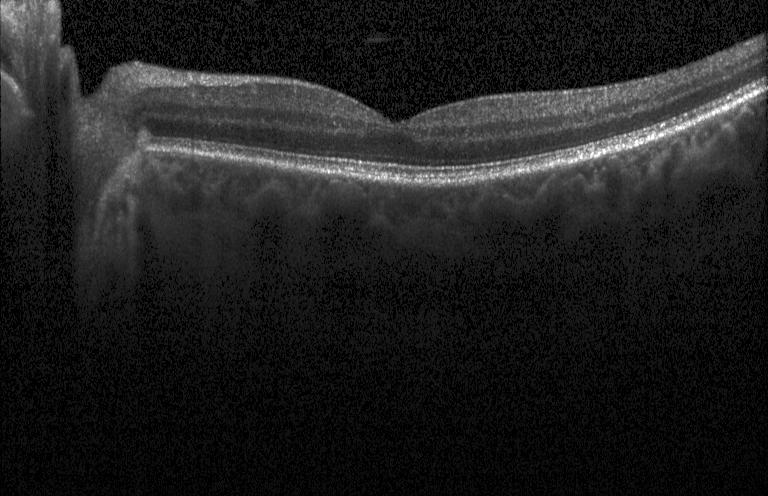 Finding: neither choroidal neovascularization, diabetic macular edema, nor drusen.